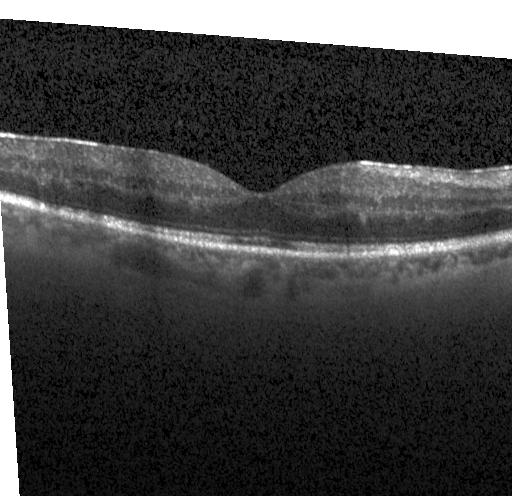

Macular OCT: neither choroidal neovascularization, diabetic macular edema, nor drusen.